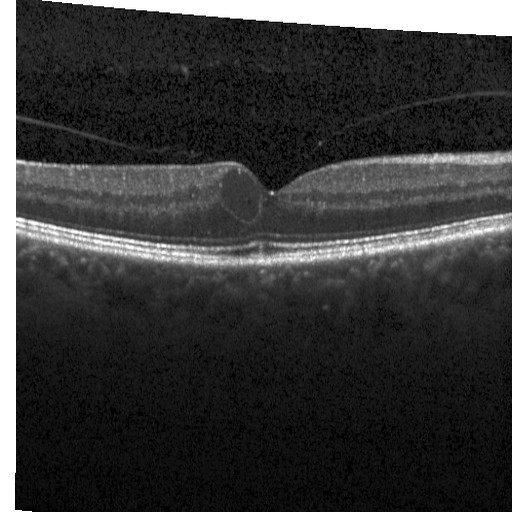 Finding: diabetic macular edema.